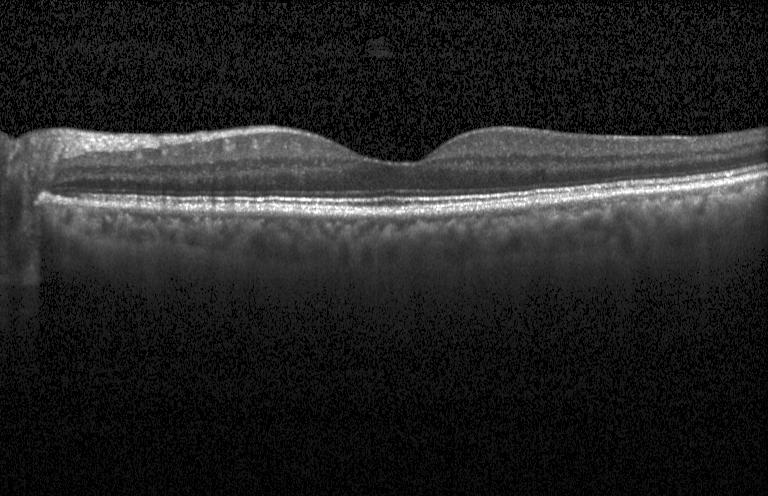 OCT line scan
This B-scan demonstrates no evidence of choroidal neovascularization, diabetic macular edema, or drusen.